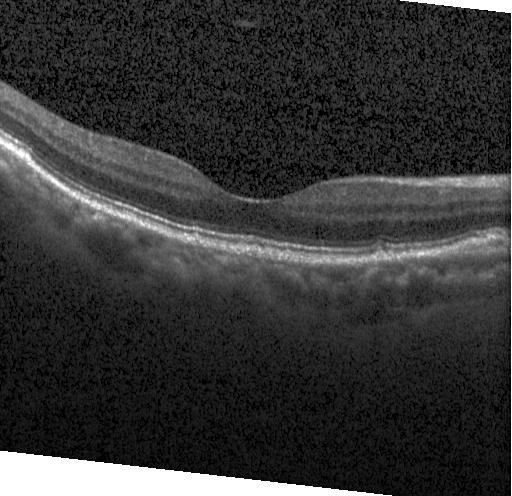 Spectral-domain optical coherence tomography; acquired on a Heidelberg Spectralis; fovea-centered; optical coherence tomography scan — Impression: no choroidal neovascularization, diabetic macular edema, or drusen.